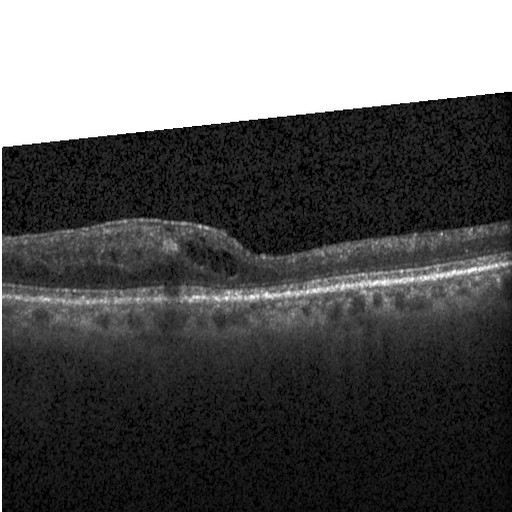
Retinal OCT cross-section showing diabetic macular edema.